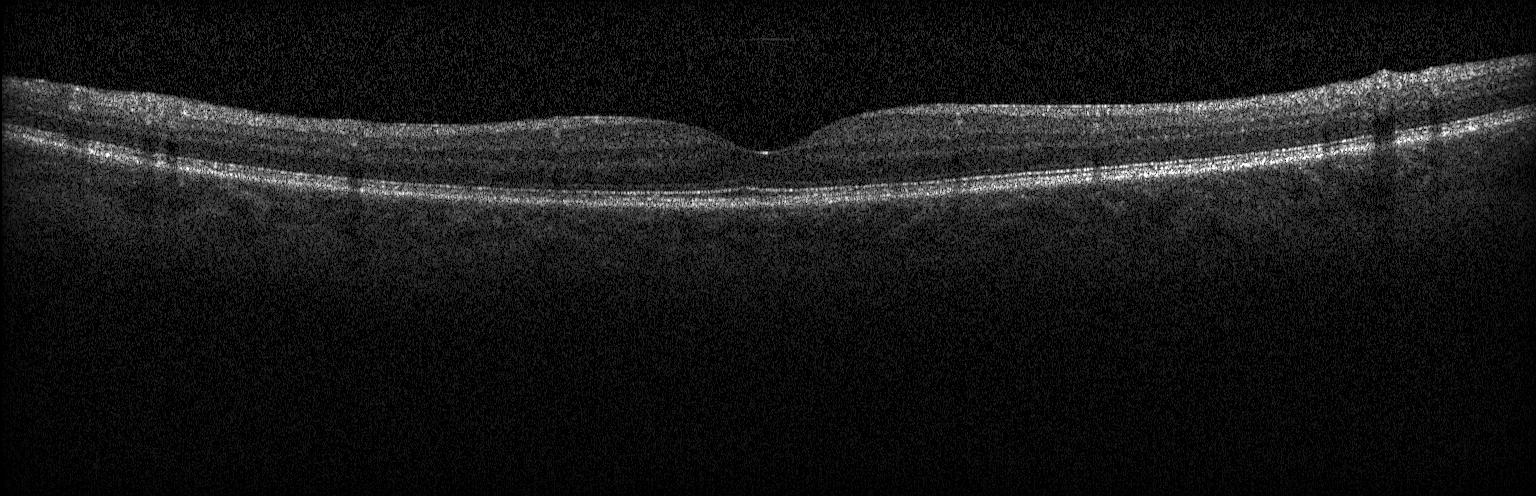
Retinal OCT cross-section — The scan shows neither choroidal neovascularization, diabetic macular edema, nor drusen.